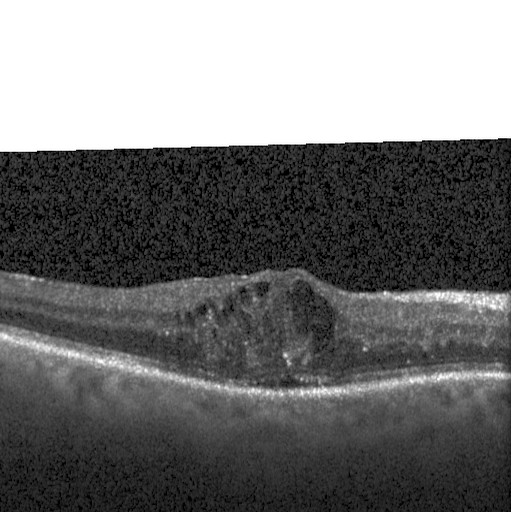

Heidelberg Spectralis, optical coherence tomography scan. Diabetic macular edema (DME).